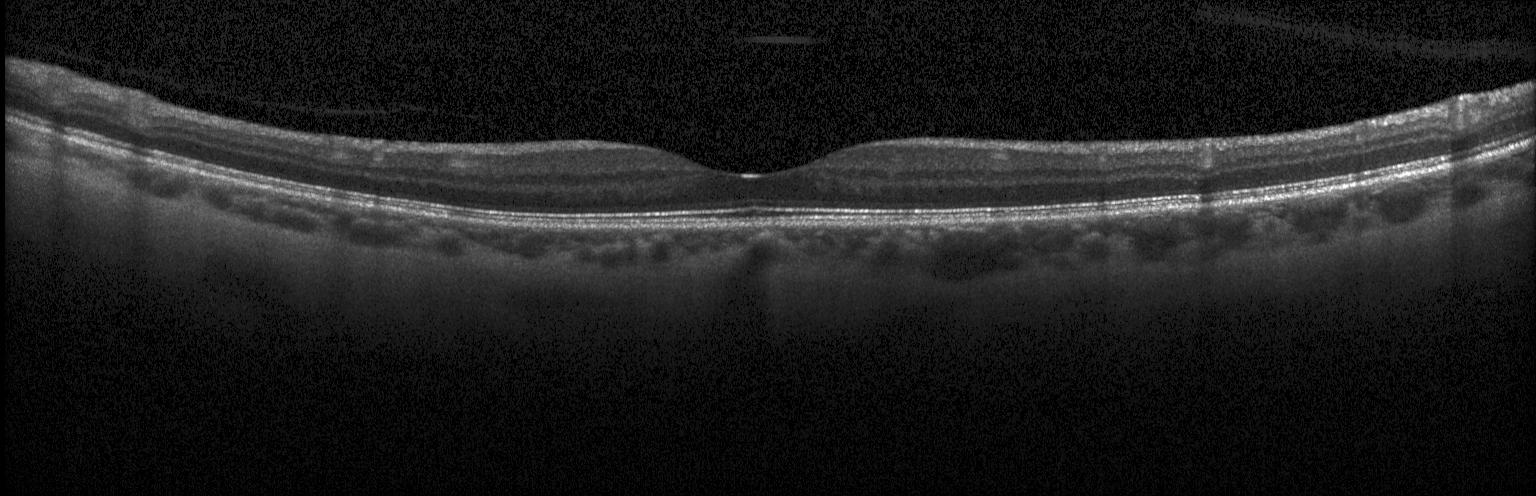

Macular OCT demonstrating no choroidal neovascularization, no diabetic macular edema, and no drusen.